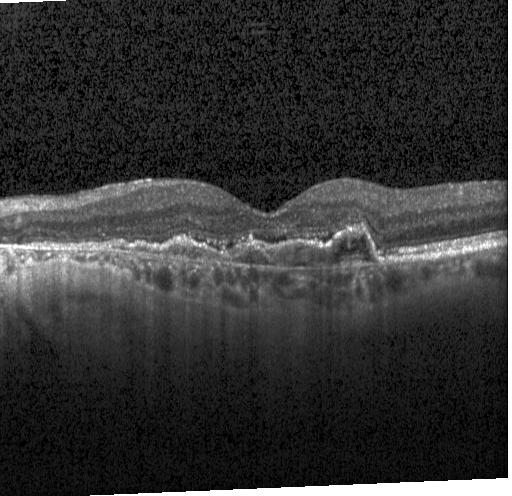
OCT finding: a choroidal neovascular membrane.